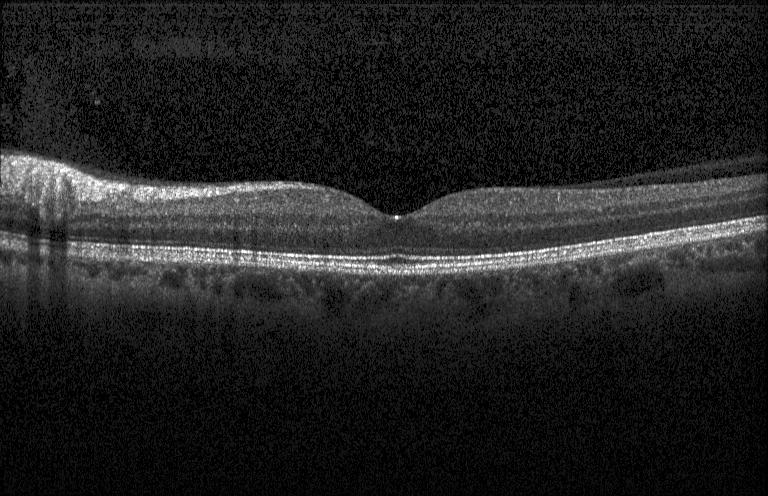

OCT B-scan.
No choroidal neovascularization, no diabetic macular edema, and no drusen.